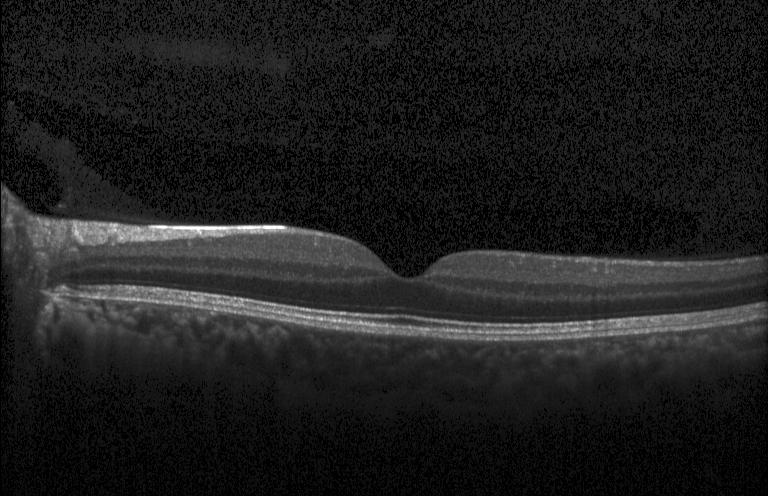

Finding: no evidence of CNV, DME, or drusen.